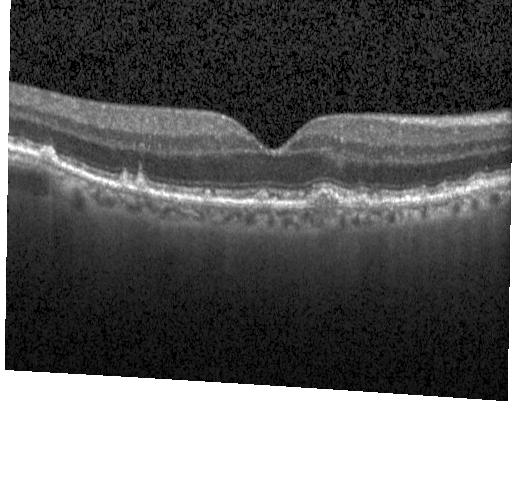
Impression: multiple drusen.